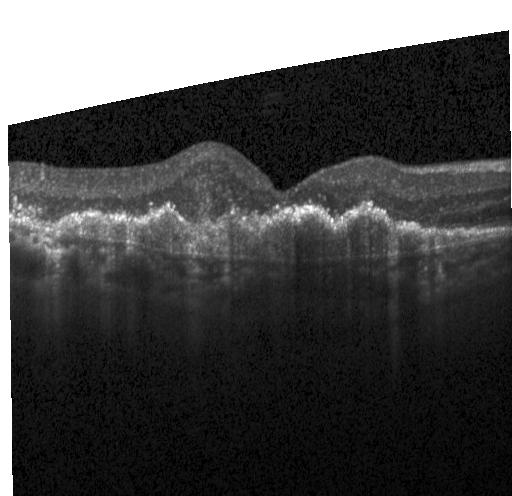 Optical coherence tomography B-scan — Diagnosis: a choroidal neovascular membrane.